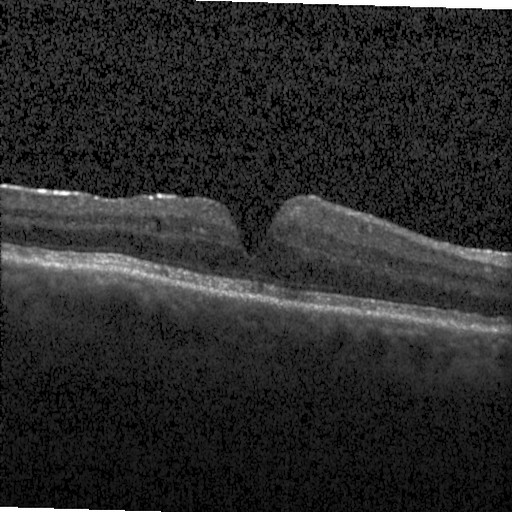 Optical coherence tomography B-scan. Impression: DME.